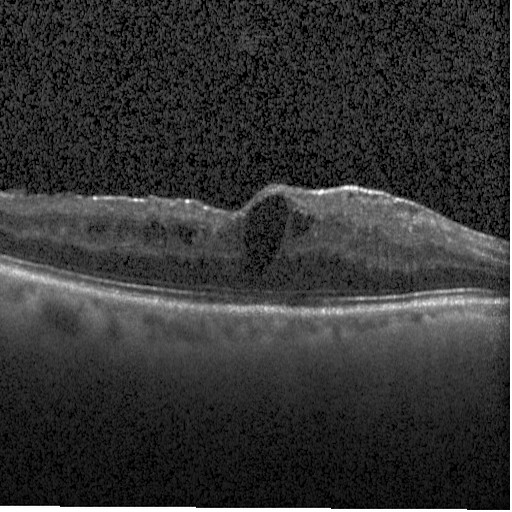

Diagnosis: diabetic macular edema (DME).